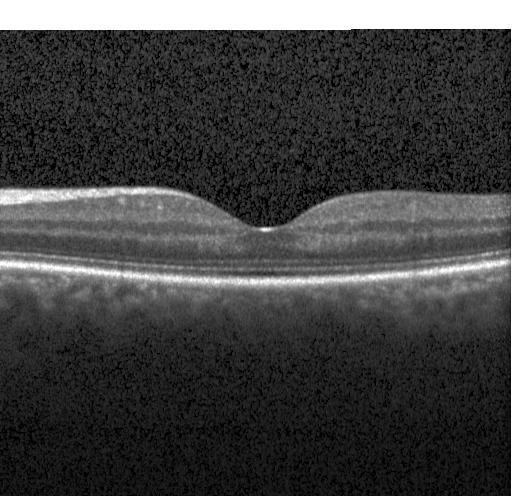 Retinal OCT B-scan · centered on the fovea · acquired on a Heidelberg Spectralis · spectral-domain OCT — Assessment: no evidence of CNV, DME, or drusen.